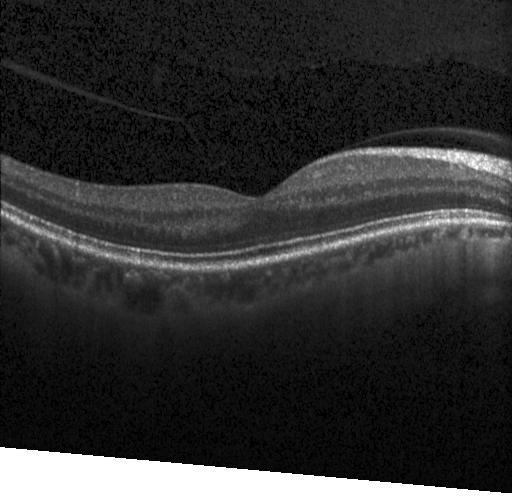 Optical coherence tomography B-scan — Impression: no choroidal neovascularization, diabetic macular edema, or drusen.